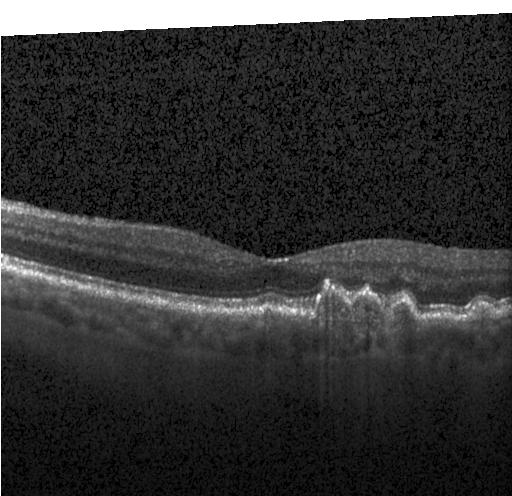

Optical coherence tomography B-scan. Impression: drusen.